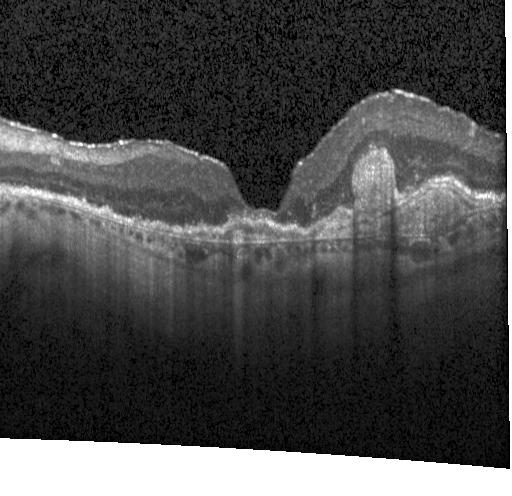 Instrument: Heidelberg Spectralis; optical coherence tomography B-scan; through the macula
This B-scan demonstrates a choroidal neovascular membrane.